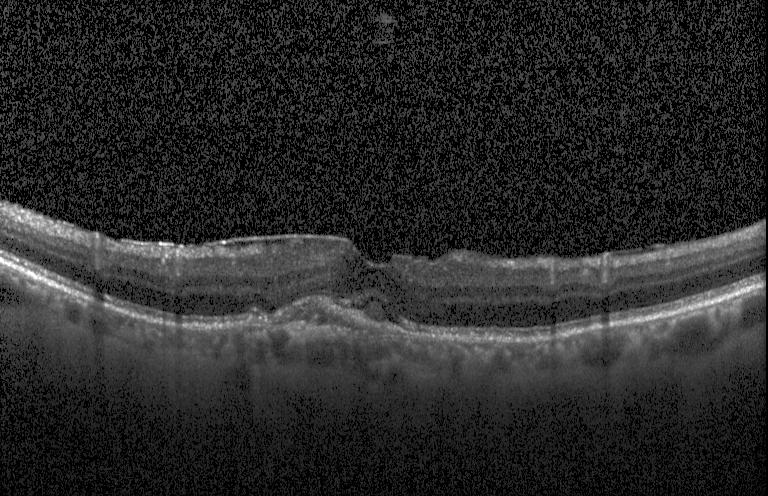 Acquired on a Heidelberg Spectralis. Through the macula. Retinal OCT B-scan
Assessment: a choroidal neovascular membrane.